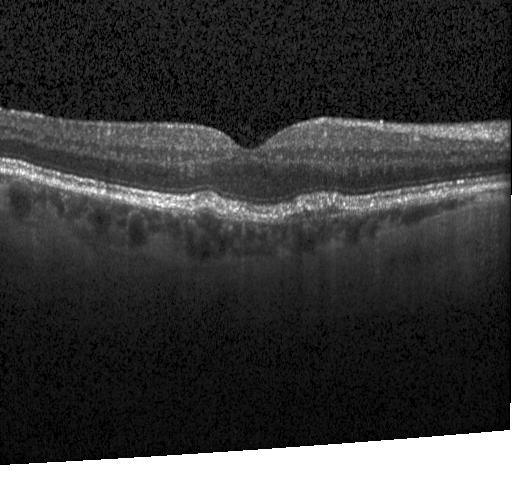 Optical coherence tomography scan, SD-OCT, Heidelberg Spectralis.
Finding: sub-RPE drusenoid deposits.